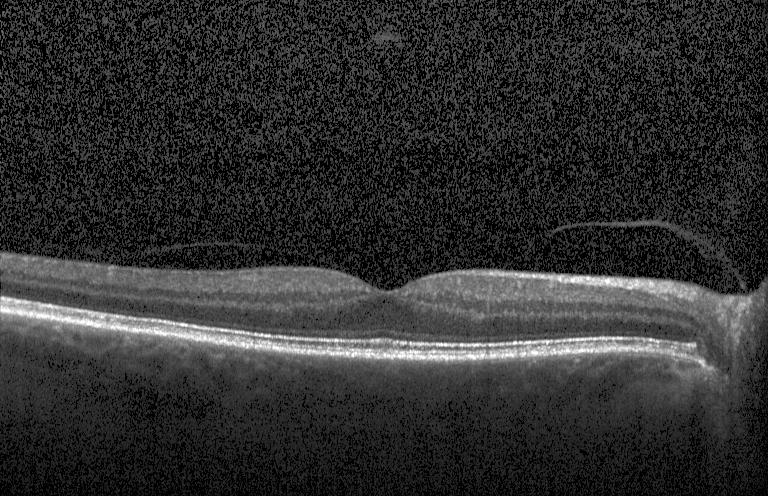 OCT B-scan showing no evidence of choroidal neovascularization, diabetic macular edema, or drusen.